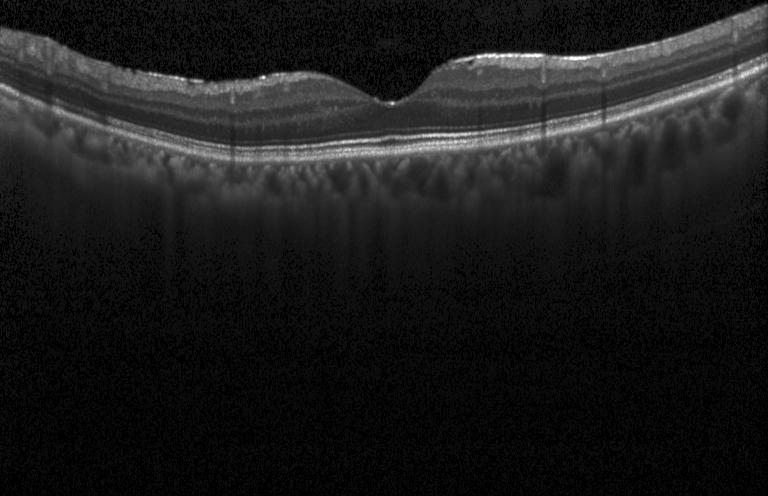

OCT B-scan showing no choroidal neovascularization, no diabetic macular edema, and no drusen.